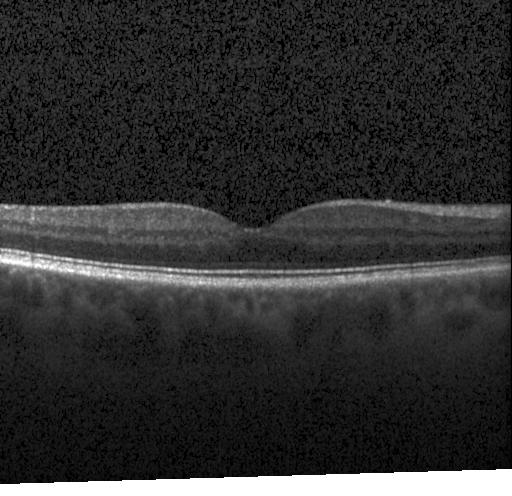

Spectral-domain OCT B-scan: no evidence of choroidal neovascularization, diabetic macular edema, or drusen.